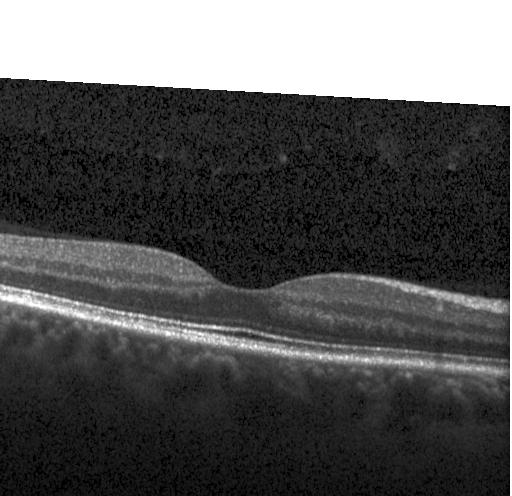
Assessment: neither CNV, DME, nor drusen.